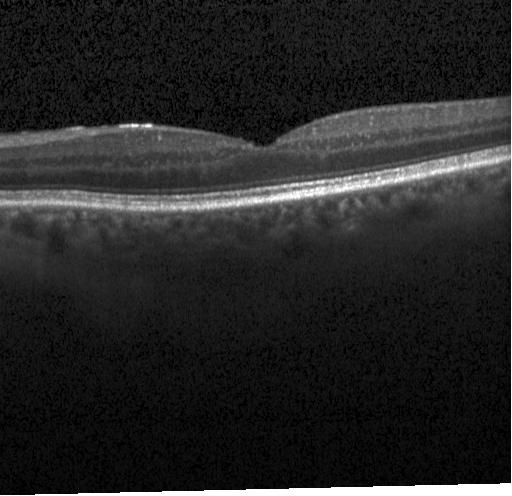
Macular scan, optical coherence tomography scan, acquired on a Heidelberg Spectralis, SD-OCT — Assessment: neither choroidal neovascularization, diabetic macular edema, nor drusen.